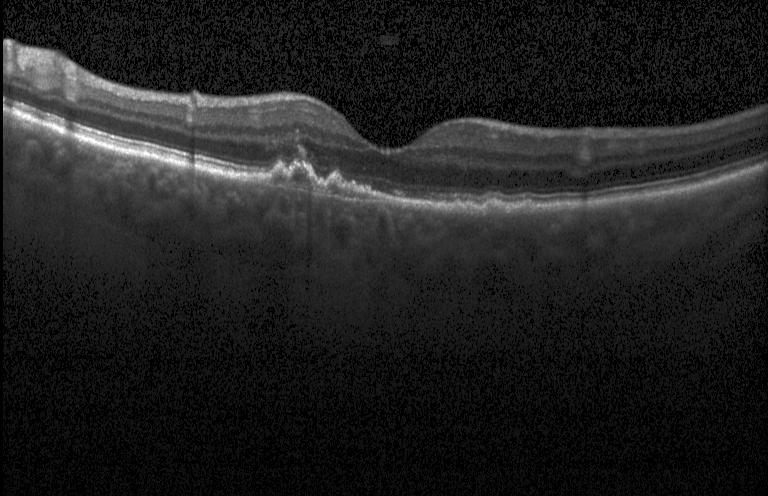 Retinal OCT cross-section showing a choroidal neovascular membrane.